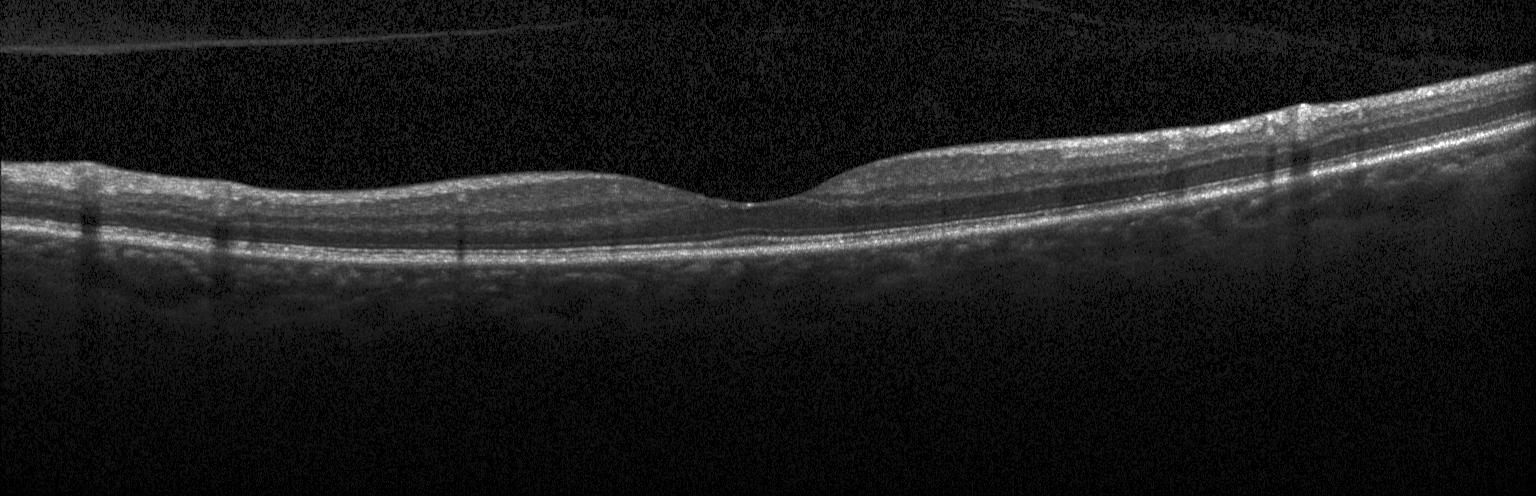
The scan shows neither CNV, DME, nor drusen.